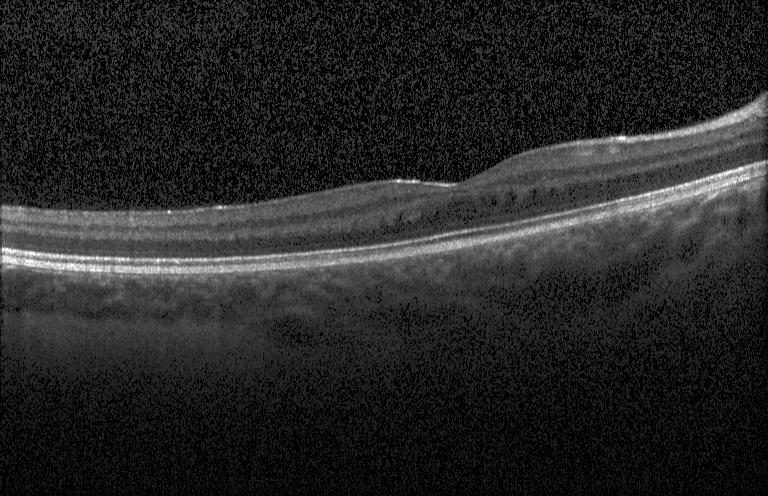 Macular OCT demonstrating no choroidal neovascularization, diabetic macular edema, or drusen.